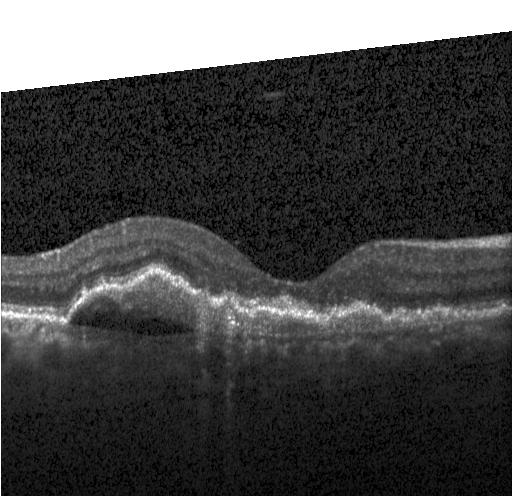

SD-OCT, retinal OCT B-scan — The scan shows a choroidal neovascular membrane.